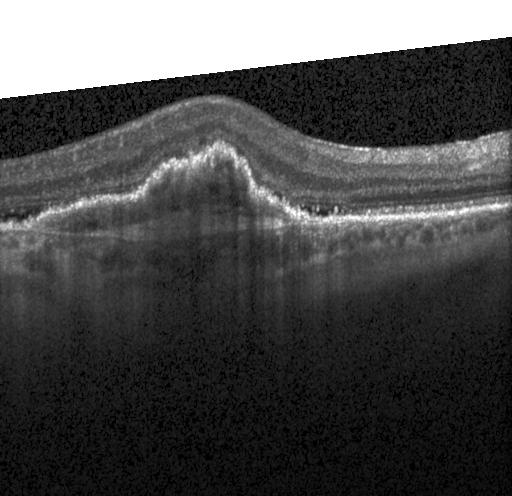 Finding: a choroidal neovascular membrane.